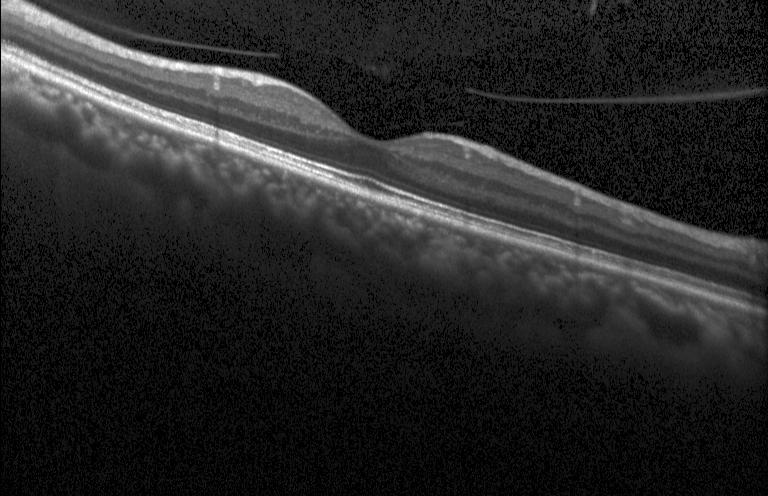 Impression: neither choroidal neovascularization, diabetic macular edema, nor drusen.